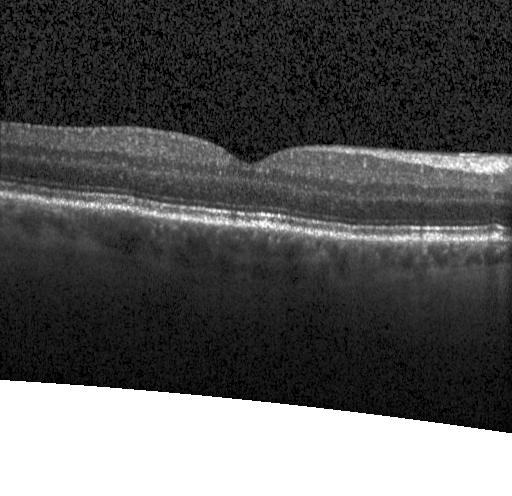

Spectral-domain OCT · OCT line scan · acquired on a Heidelberg Spectralis. Diagnosis: neither CNV, DME, nor drusen.